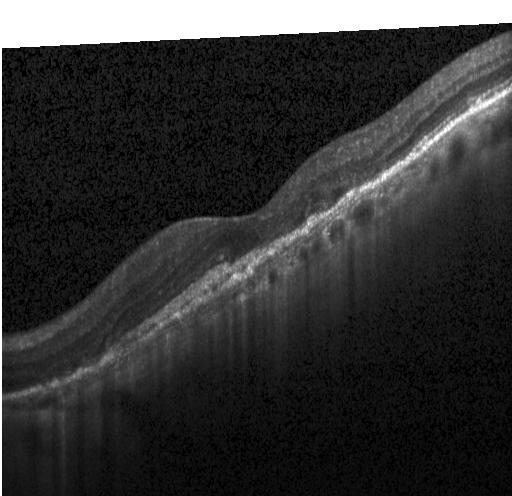 Dx: a choroidal neovascular membrane.